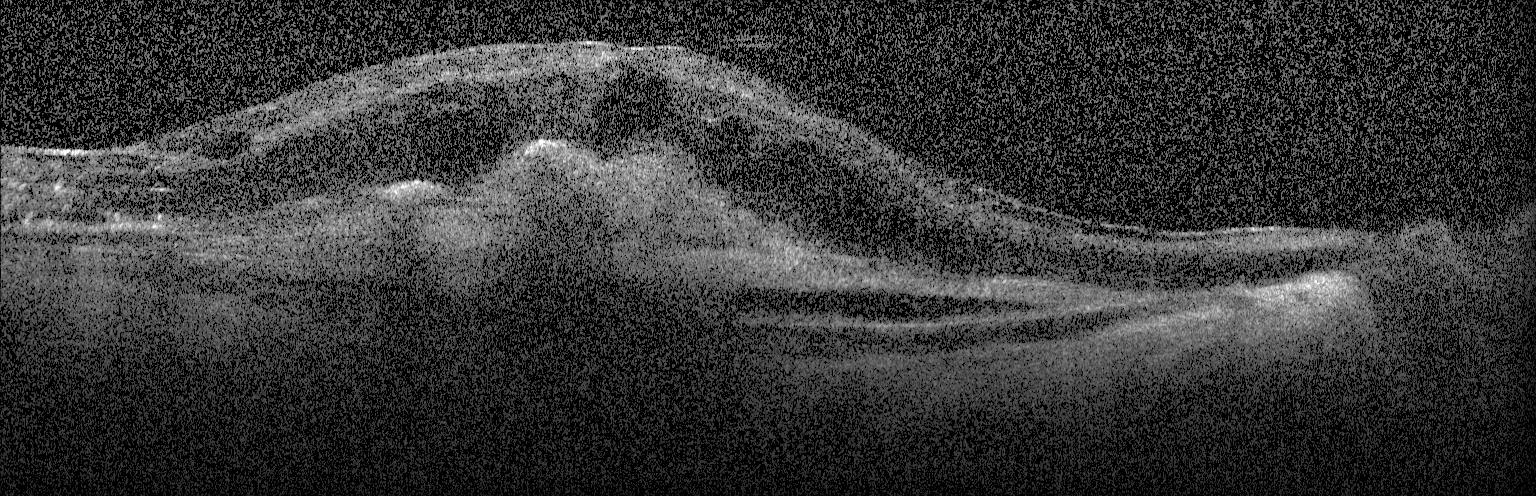 Diagnosis: a choroidal neovascular membrane.